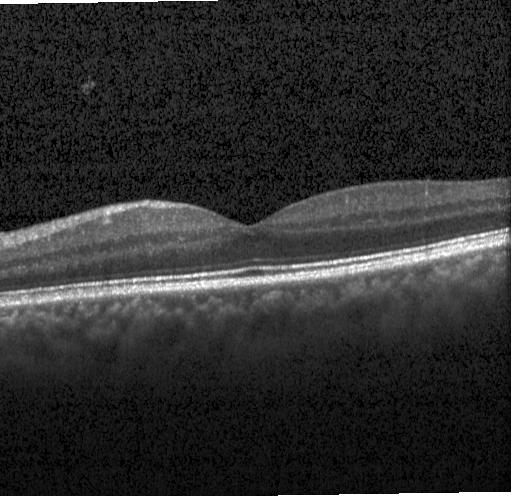
Macular OCT demonstrating no choroidal neovascularization, no diabetic macular edema, and no drusen.